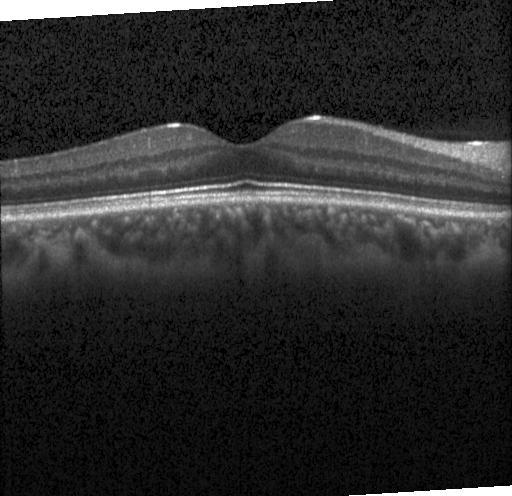 Retinal OCT cross-section showing no evidence of choroidal neovascularization, diabetic macular edema, or drusen.